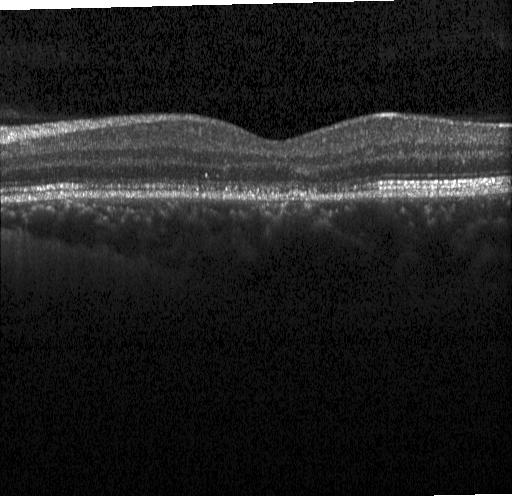
Retinal OCT B-scan. This B-scan demonstrates no CNV, DME, or drusen.